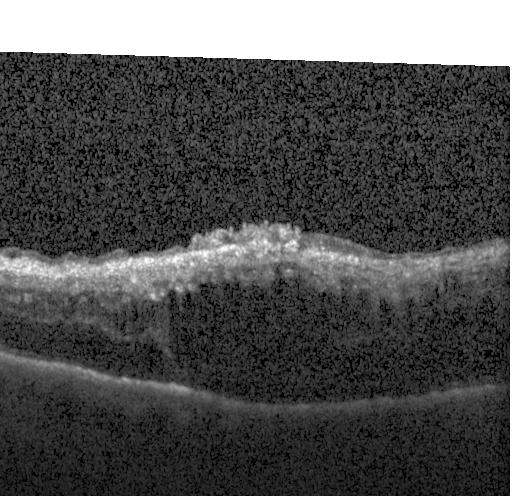
Optical coherence tomography B-scan. Impression: diabetic macular edema.